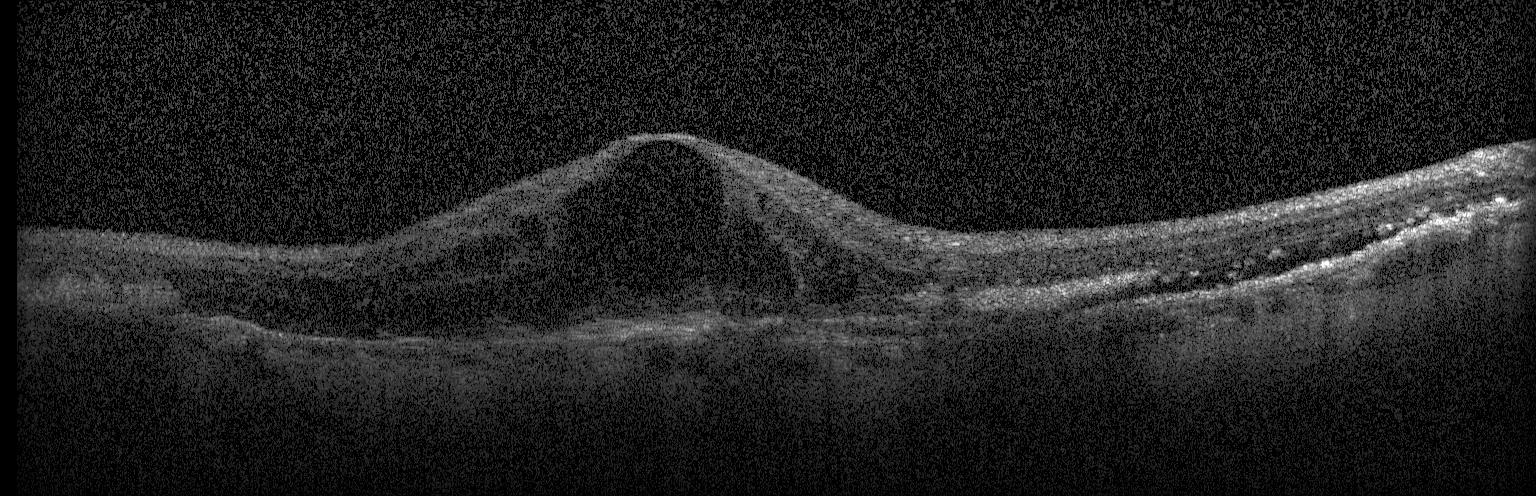
Heidelberg Spectralis OCT system. Retinal OCT B-scan. SD-OCT.
This B-scan demonstrates a choroidal neovascular membrane.